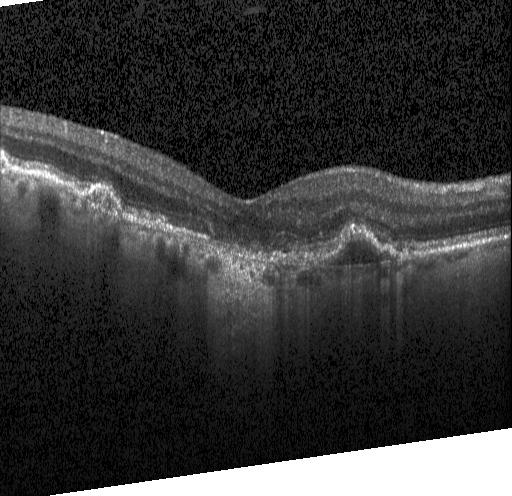

OCT B-scan
Choroidal neovascularization (CNV).